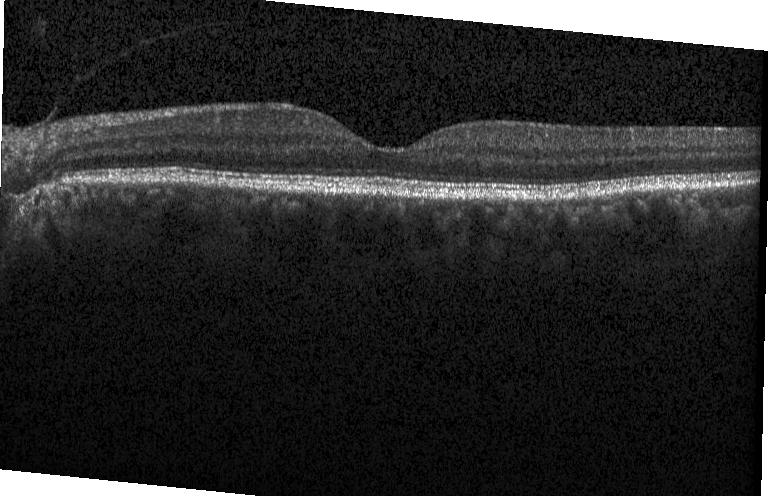
Dx: no evidence of choroidal neovascularization, diabetic macular edema, or drusen.